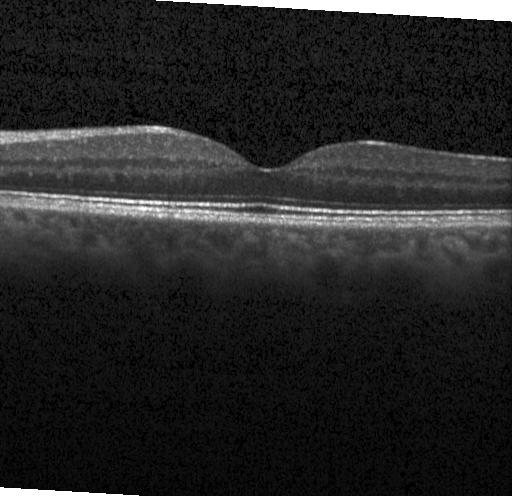

Fovea-centered; acquired on a Heidelberg Spectralis; optical coherence tomography scan.
OCT finding: neither choroidal neovascularization, diabetic macular edema, nor drusen.